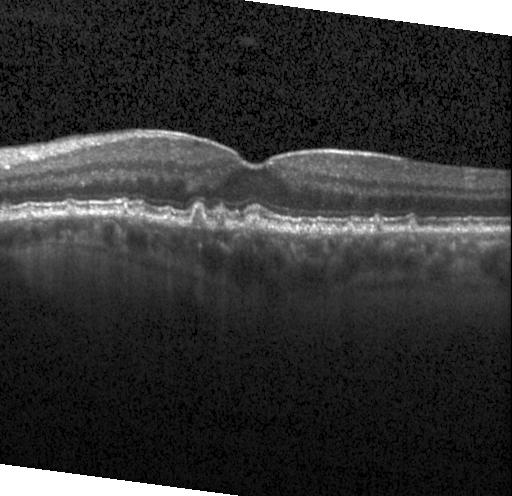
The scan shows multiple drusen.